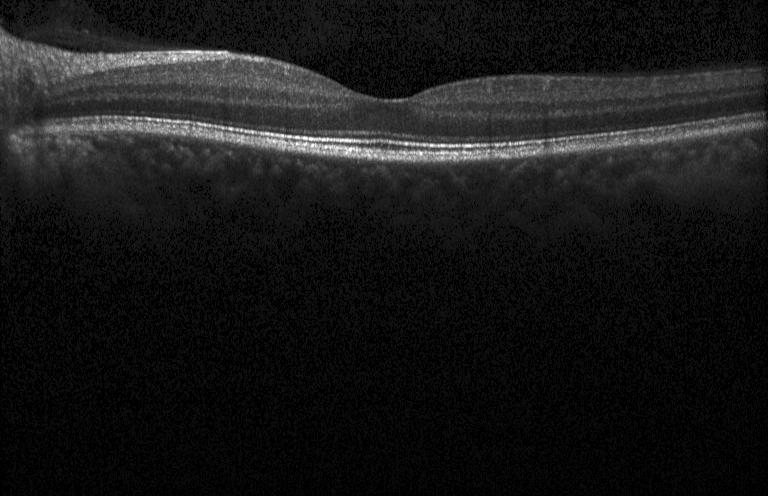
Spectral-domain optical coherence tomography; macular scan; acquired on a Heidelberg Spectralis; optical coherence tomography B-scan.
Impression: no choroidal neovascularization, diabetic macular edema, or drusen.